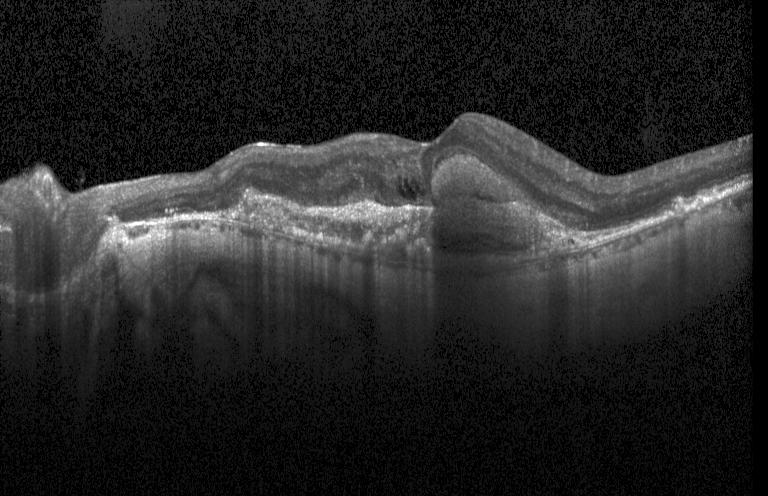

Finding: choroidal neovascularization (CNV).